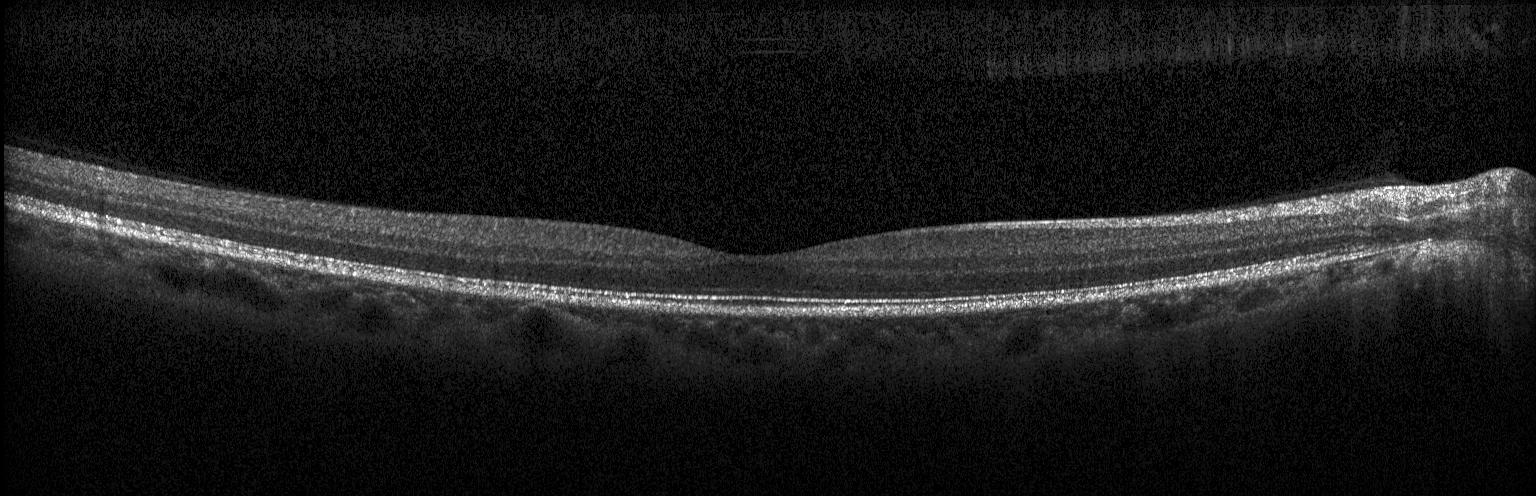
The scan shows no CNV, DME, or drusen.